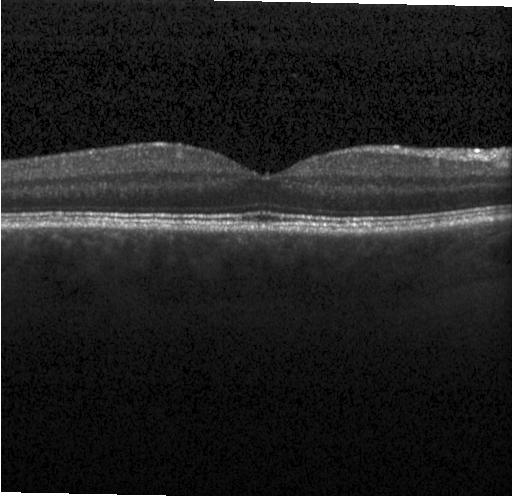 OCT finding: neither CNV, DME, nor drusen.